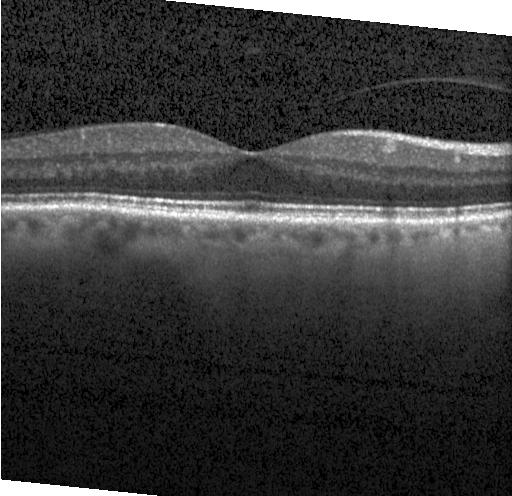

Macular OCT demonstrating no evidence of choroidal neovascularization, diabetic macular edema, or drusen.